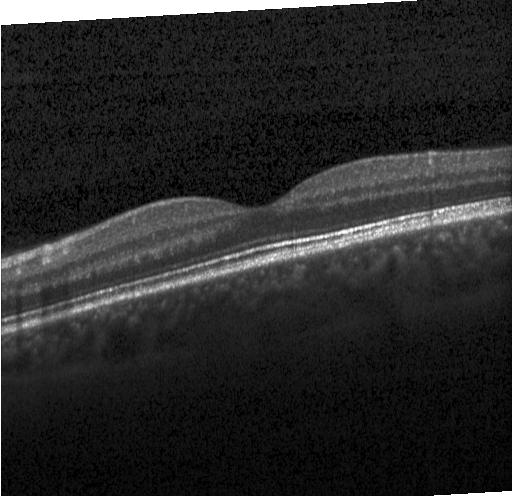
OCT B-scan. Spectral-domain optical coherence tomography. Through the macula. Dx: no choroidal neovascularization, diabetic macular edema, or drusen.